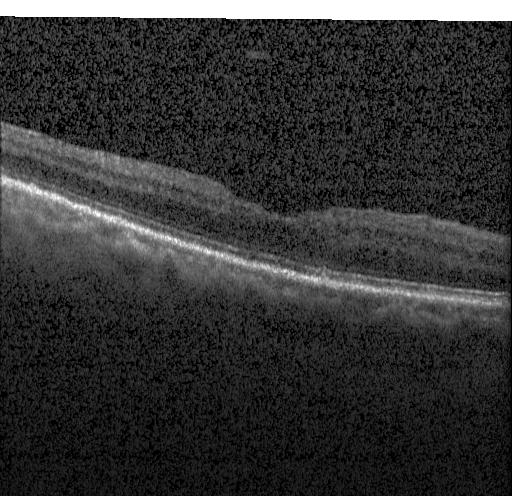
Horizontal scan through the fovea · spectral-domain OCT · OCT B-scan.
Impression: no evidence of choroidal neovascularization, diabetic macular edema, or drusen.